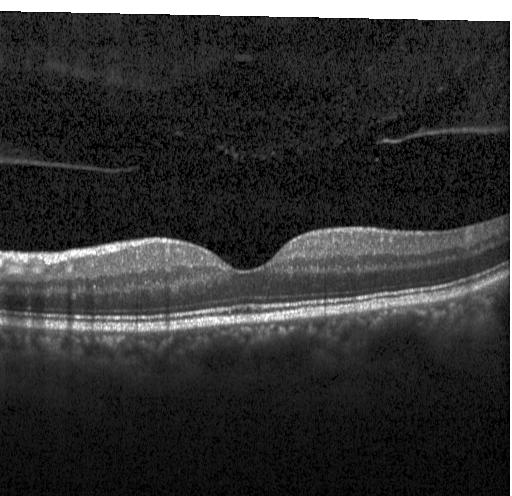

Acquired on a Heidelberg Spectralis; retinal OCT B-scan; spectral-domain optical coherence tomography; fovea-centered. Macular OCT: no evidence of choroidal neovascularization, diabetic macular edema, or drusen.